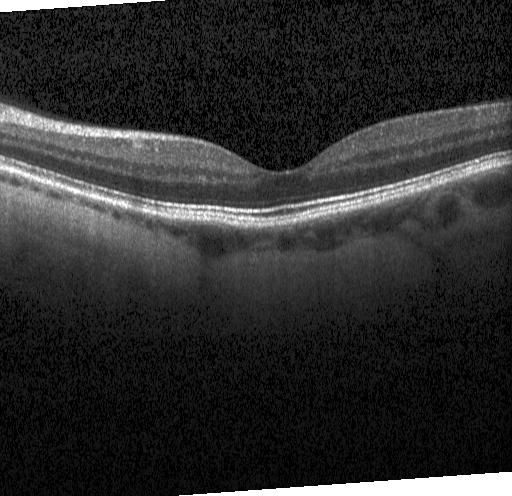

OCT line scan. Assessment: no evidence of CNV, DME, or drusen.